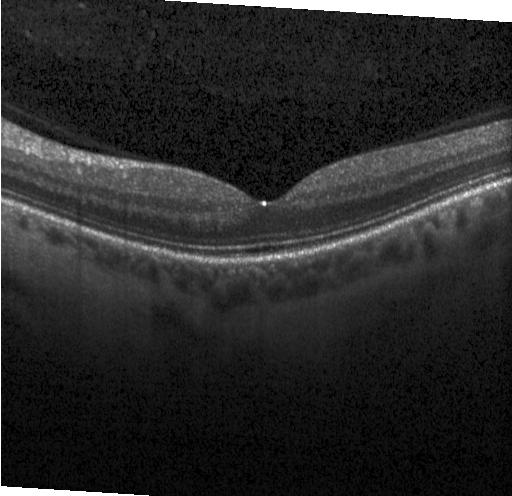

Heidelberg Spectralis OCT system · optical coherence tomography scan — No choroidal neovascularization, no diabetic macular edema, and no drusen.